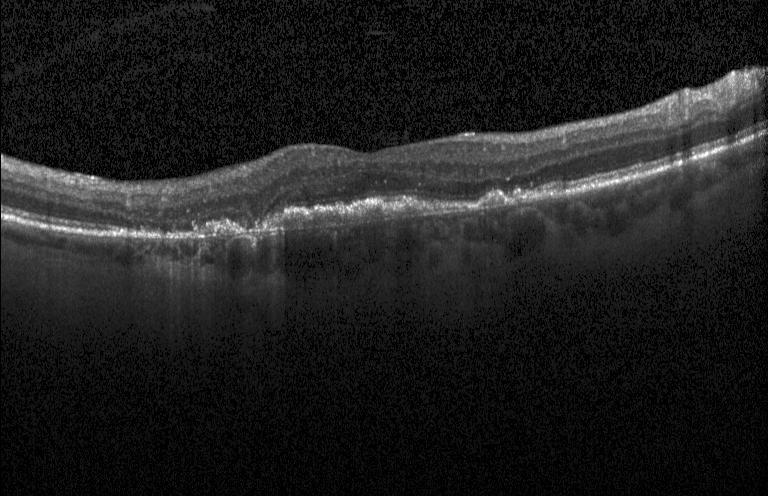
Finding: a choroidal neovascular membrane.